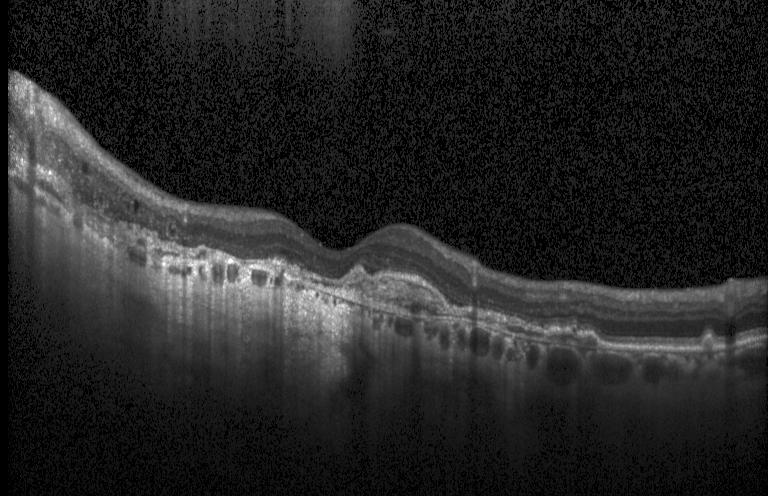
Centered on the fovea, spectral-domain optical coherence tomography, retinal OCT B-scan, instrument: Heidelberg Spectralis.
A choroidal neovascular membrane.